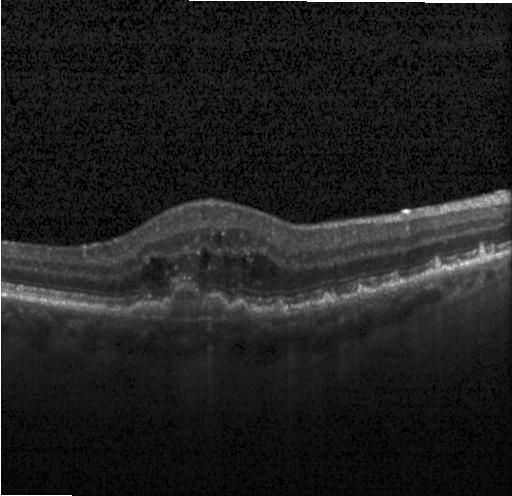
OCT B-scan showing a choroidal neovascular membrane.